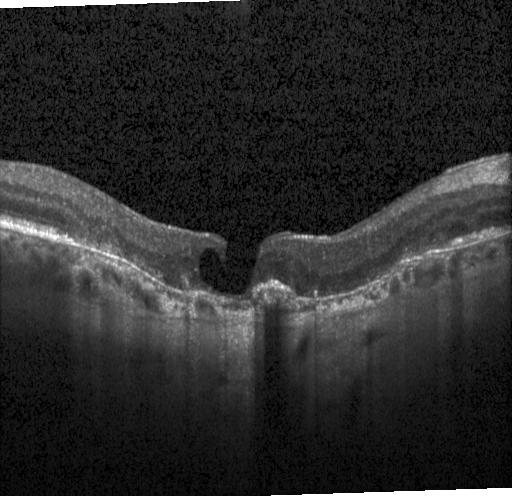
Optical coherence tomography B-scan · instrument: Heidelberg Spectralis · centered on the fovea
Choroidal neovascularization (CNV).